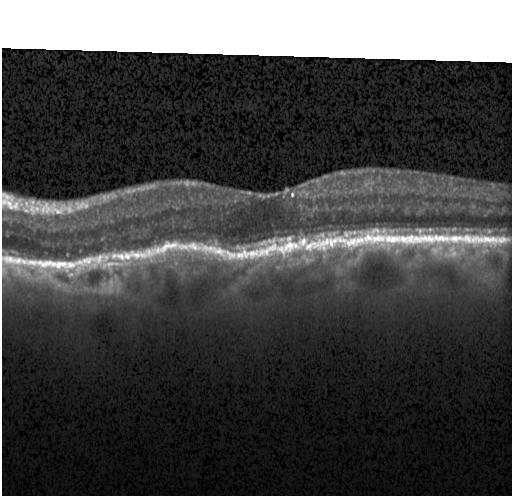 Optical coherence tomography B-scan. Impression: a choroidal neovascular membrane.